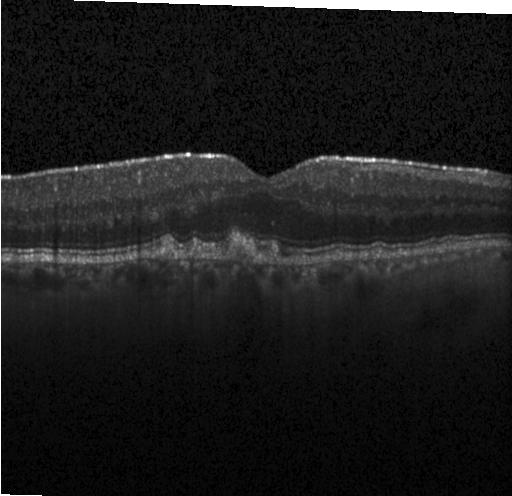 Optical coherence tomography B-scan · horizontal scan through the fovea
Impression: multiple drusen.